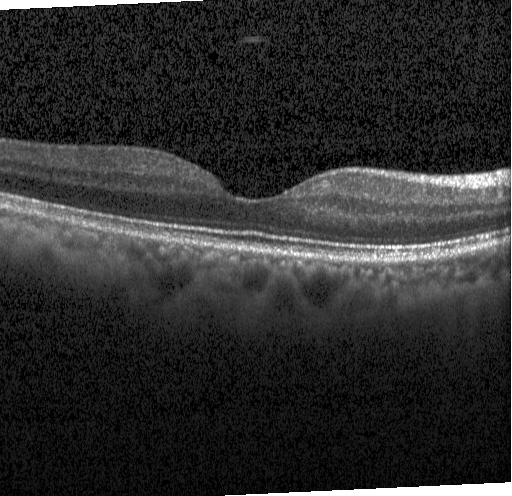

Macular scan. OCT B-scan. No evidence of choroidal neovascularization, diabetic macular edema, or drusen.